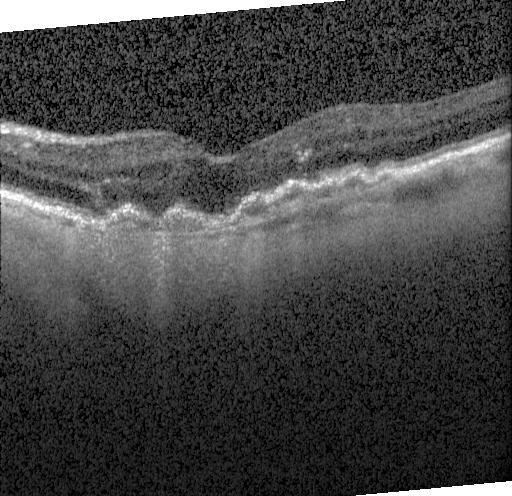 Optical coherence tomography scan — Assessment: choroidal neovascularization.